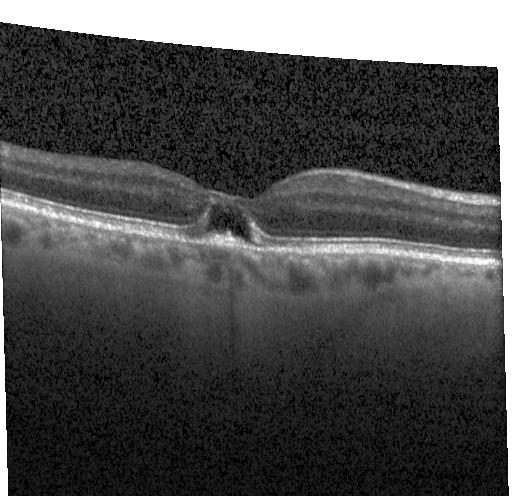
Diagnosis: a choroidal neovascular membrane.